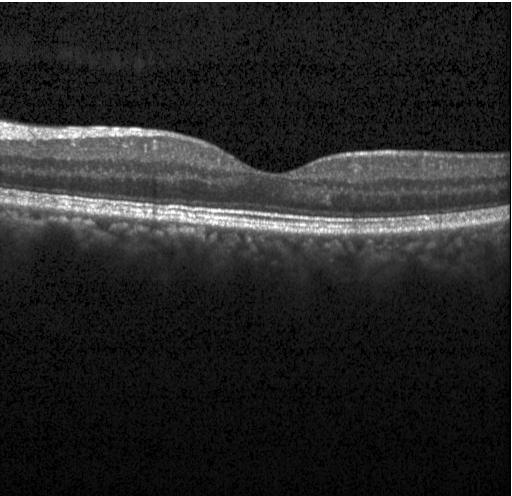 Diagnosis: no choroidal neovascularization, no diabetic macular edema, and no drusen.